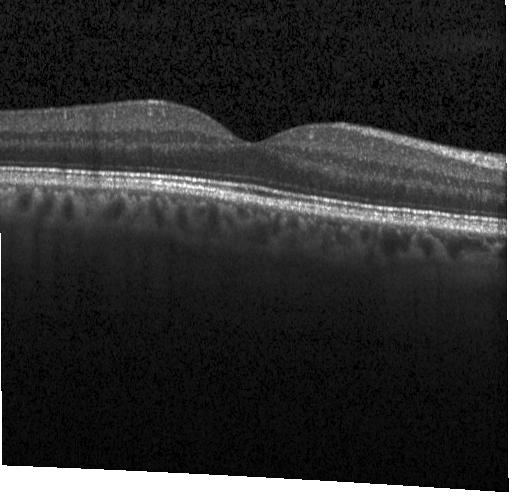
OCT scan showing neither choroidal neovascularization, diabetic macular edema, nor drusen.